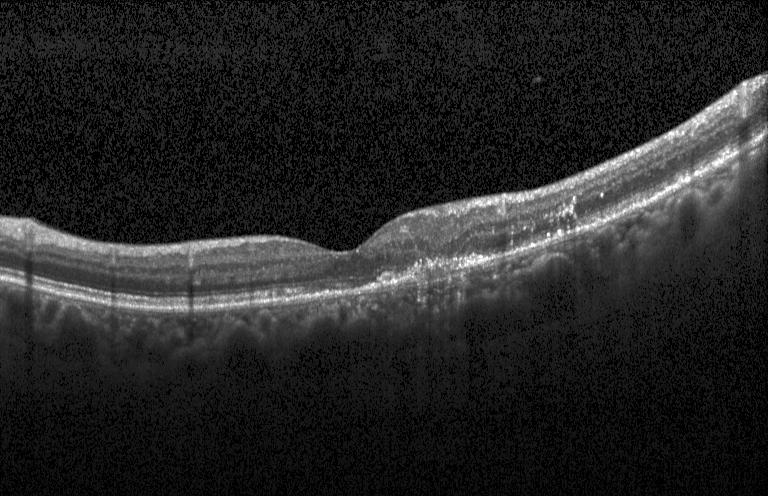

Optical coherence tomography B-scan. Impression: a choroidal neovascular membrane.